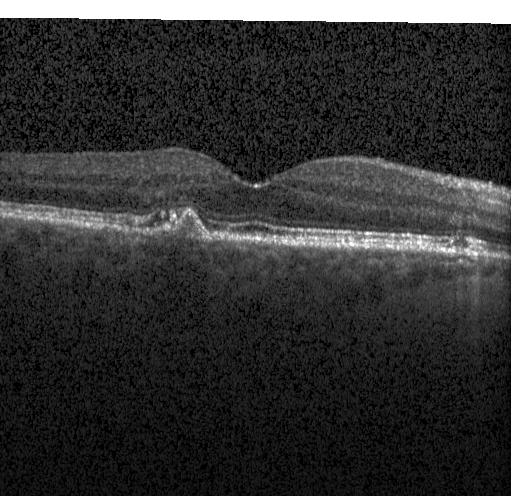 Retinal OCT cross-section showing choroidal neovascularization.